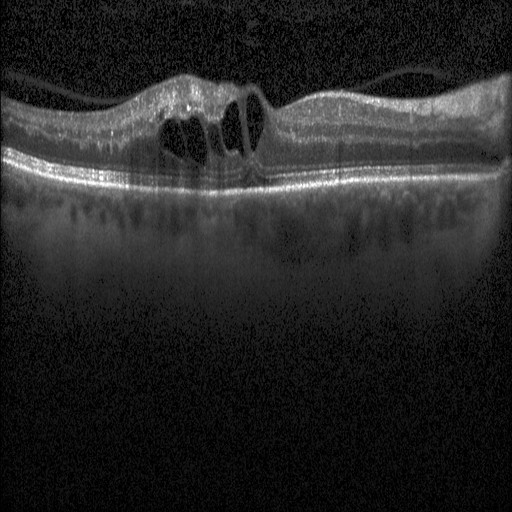
Macular OCT: DME.